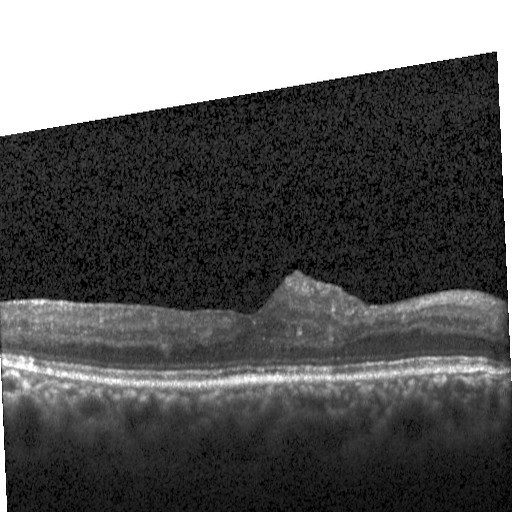

Diagnosis: diabetic macular edema.